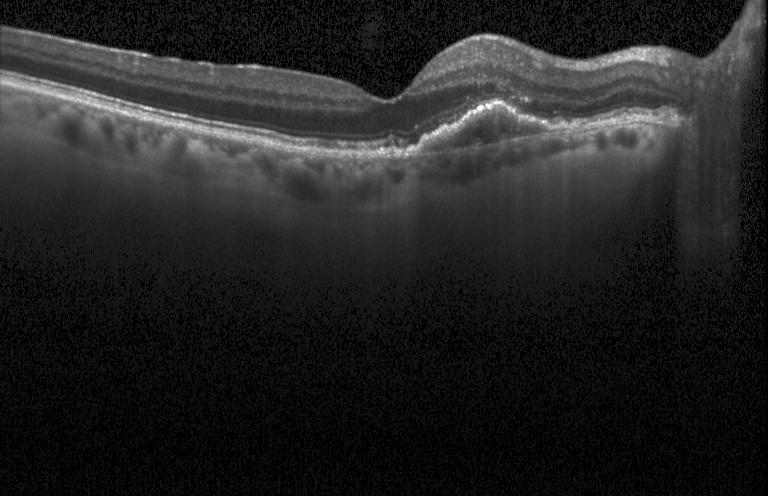
Impression: CNV.